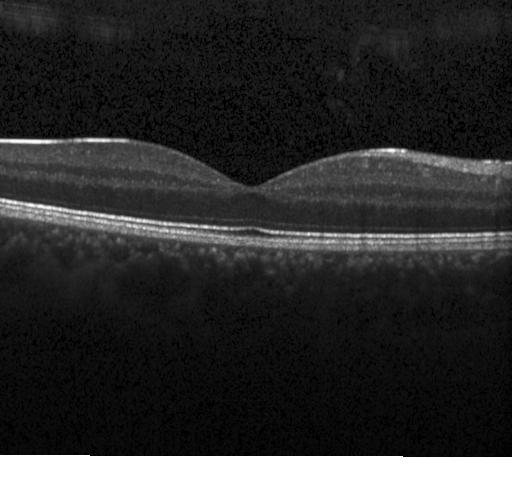 Macular OCT: no CNV, DME, or drusen.